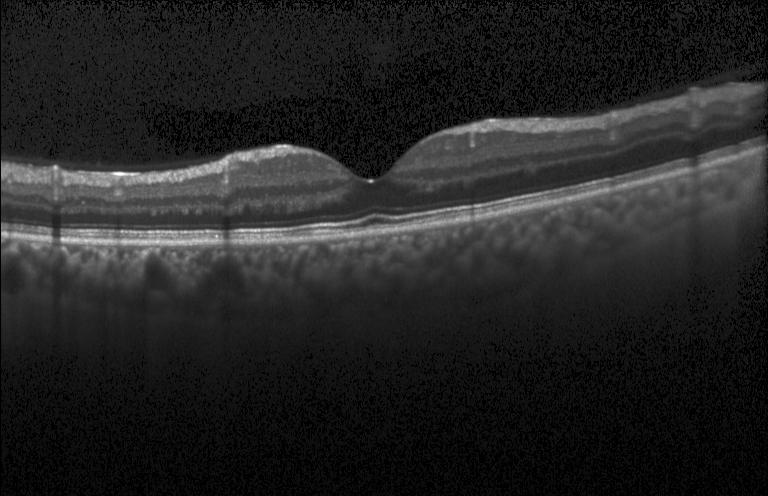 Optical coherence tomography B-scan · spectral-domain OCT · macular scan. No CNV, DME, or drusen.